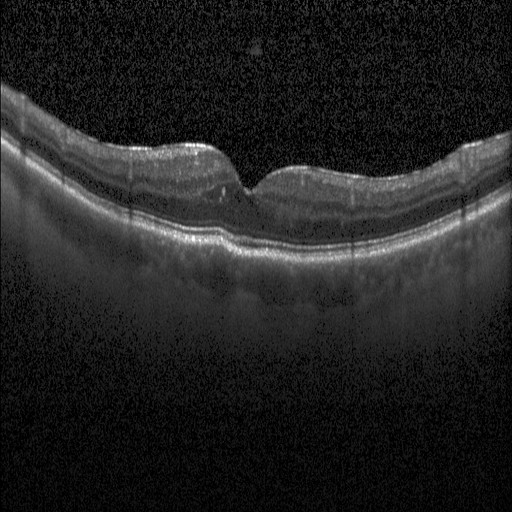

Fovea-centered. Optical coherence tomography B-scan. Spectral-domain optical coherence tomography. Heidelberg Spectralis OCT system. Finding: DME.